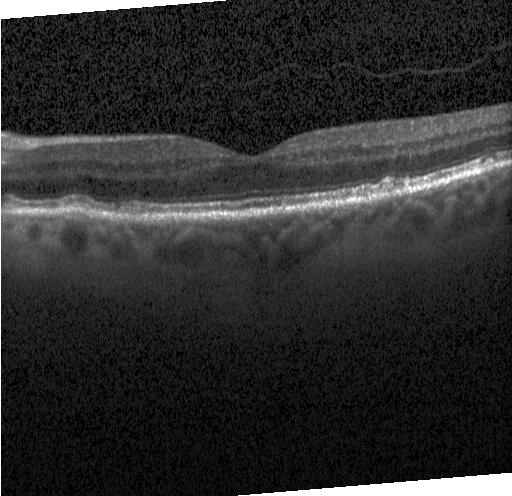

Optical coherence tomography scan, horizontal scan through the fovea, spectral-domain optical coherence tomography
Impression: sub-RPE drusenoid deposits.